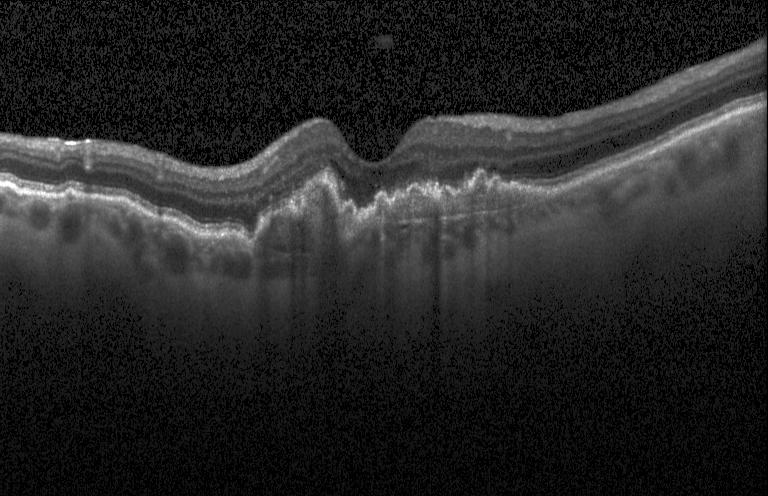

Diagnosis: CNV.